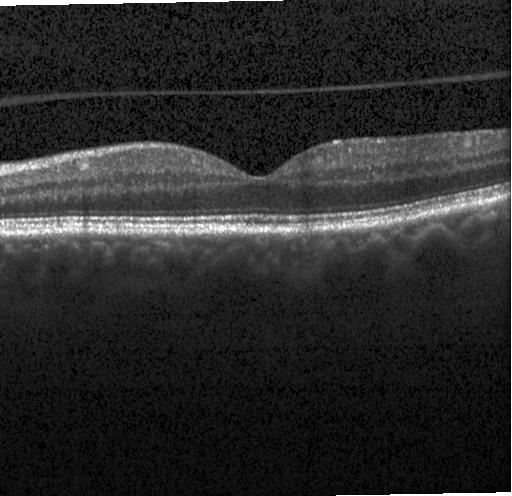
Impression: neither choroidal neovascularization, diabetic macular edema, nor drusen.